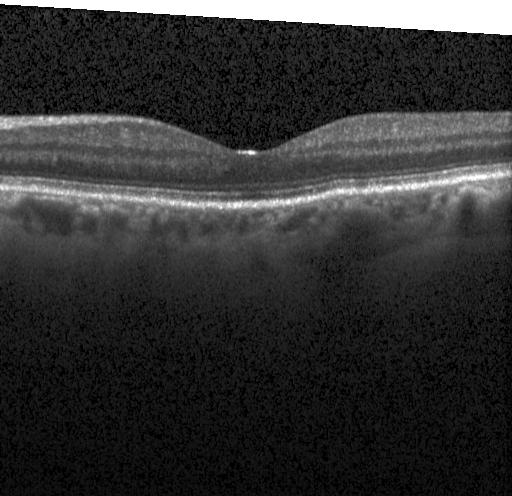

Spectral-domain optical coherence tomography, optical coherence tomography B-scan, macular scan, Heidelberg Spectralis
Finding: no CNV, DME, or drusen.